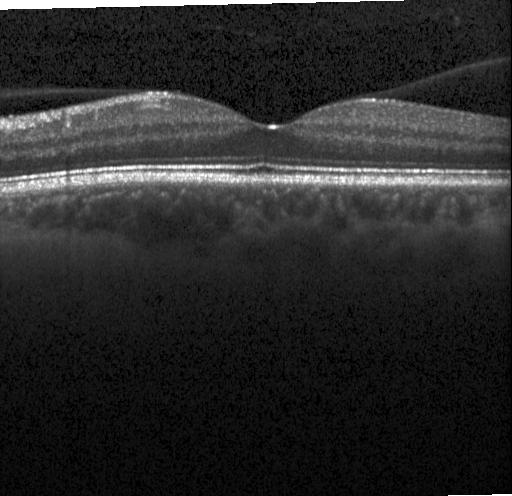

Retinal OCT cross-section showing no choroidal neovascularization, no diabetic macular edema, and no drusen.